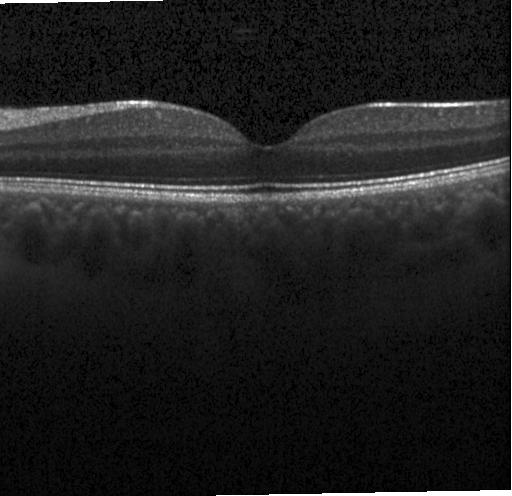

Diagnosis: no evidence of choroidal neovascularization, diabetic macular edema, or drusen.